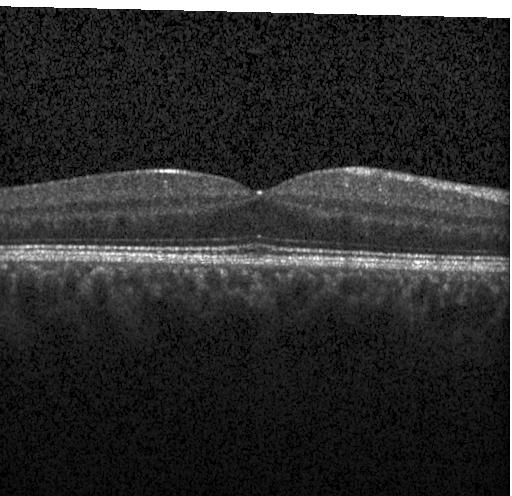

Fovea-centered; SD-OCT; optical coherence tomography scan; instrument: Heidelberg Spectralis — Impression: no CNV, no DME, and no drusen.